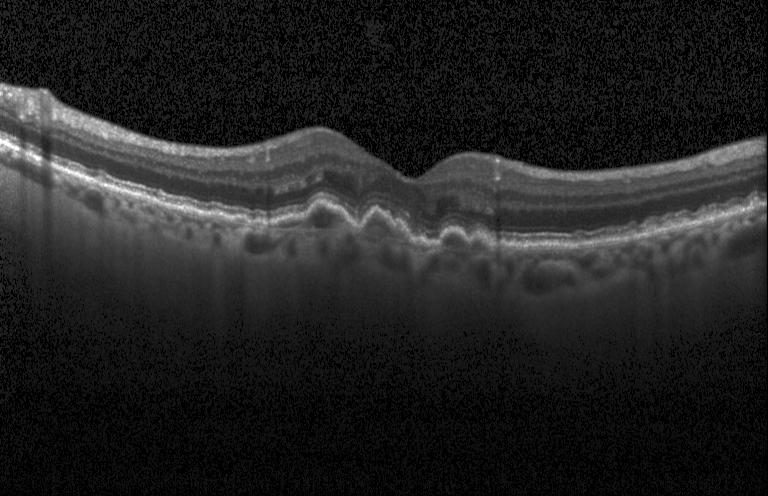

Dx: choroidal neovascularization.